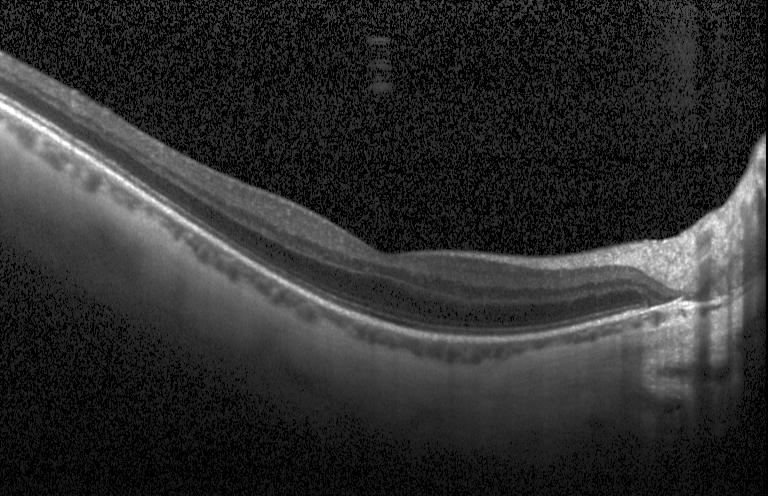 Retinal OCT cross-section · spectral-domain OCT — The scan shows no CNV, DME, or drusen.